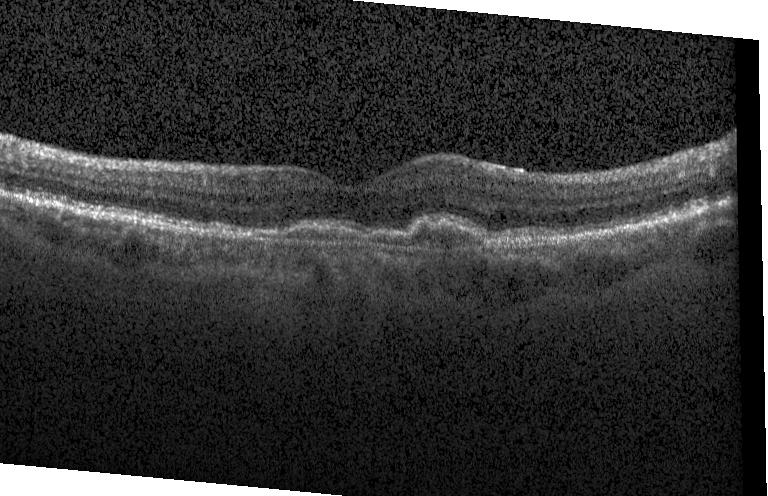

Spectral-domain OCT; retinal OCT cross-section.
This B-scan demonstrates a choroidal neovascular membrane.